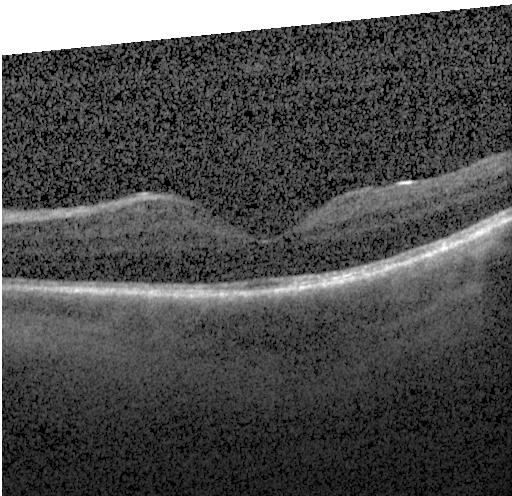

Optical coherence tomography scan. Diagnosis: no choroidal neovascularization, diabetic macular edema, or drusen.